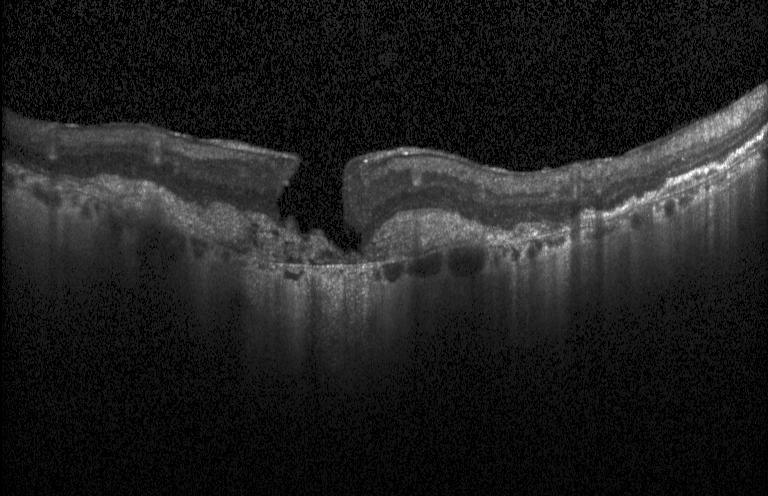
Macular OCT demonstrating CNV.